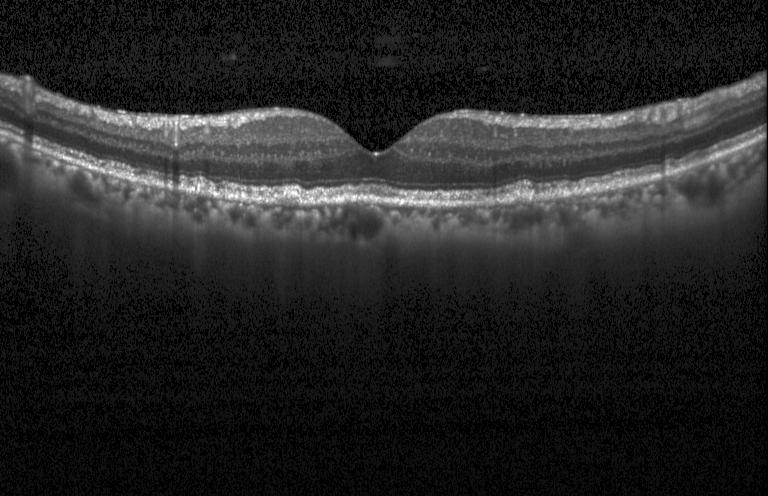

Diagnosis: multiple drusen.